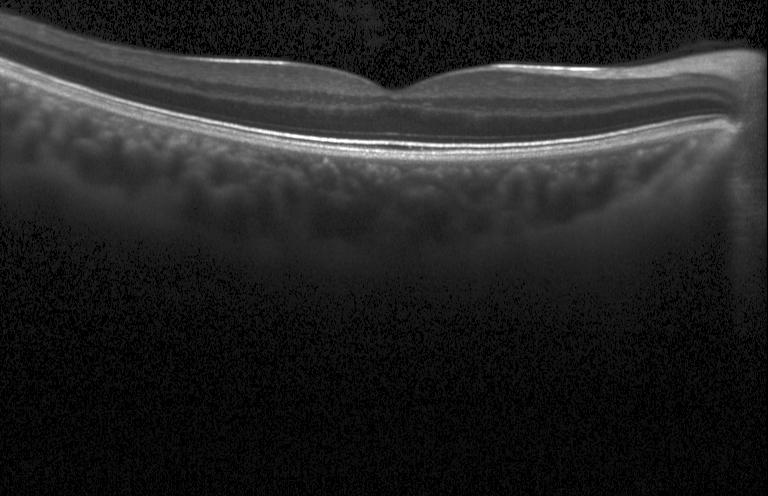 Optical coherence tomography B-scan · acquired on a Heidelberg Spectralis · spectral-domain OCT — This B-scan demonstrates no choroidal neovascularization, diabetic macular edema, or drusen.